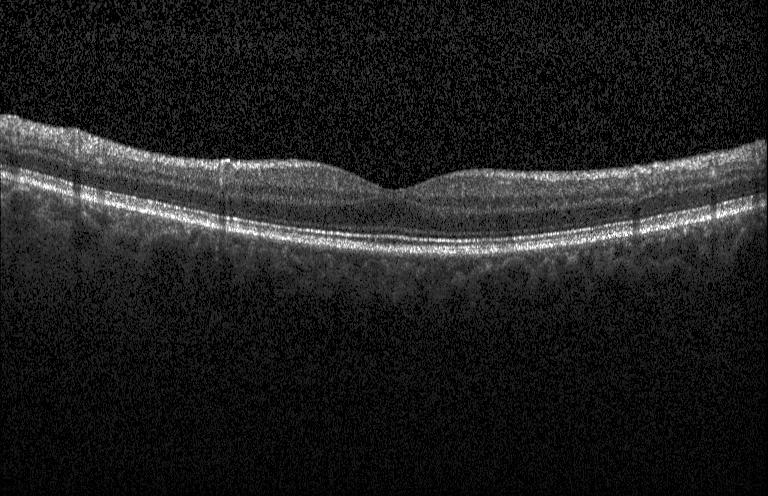
Fovea-centered. SD-OCT. Optical coherence tomography scan. Heidelberg Spectralis — No choroidal neovascularization, diabetic macular edema, or drusen.